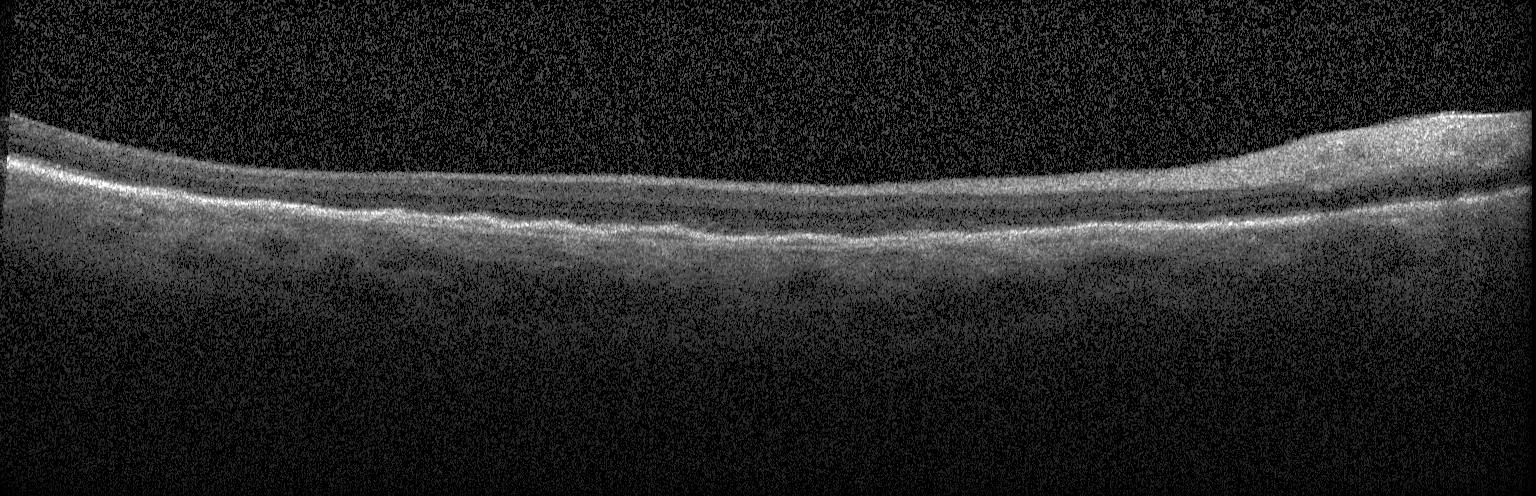
Macular OCT: choroidal neovascularization (CNV).